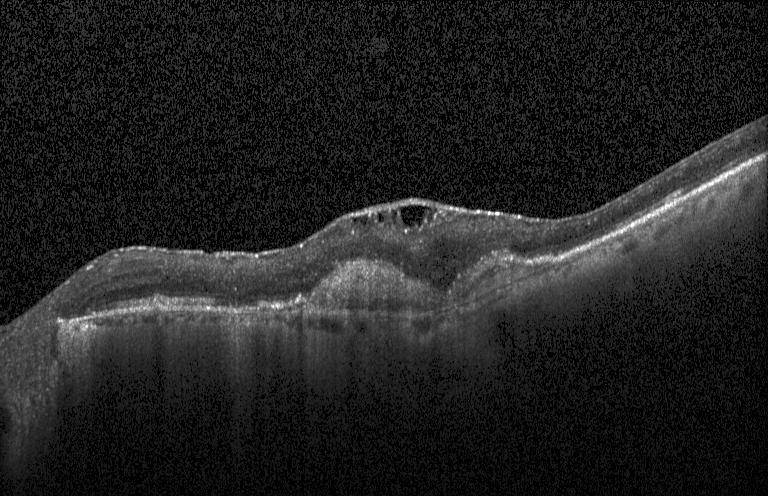
OCT scan showing choroidal neovascularization.